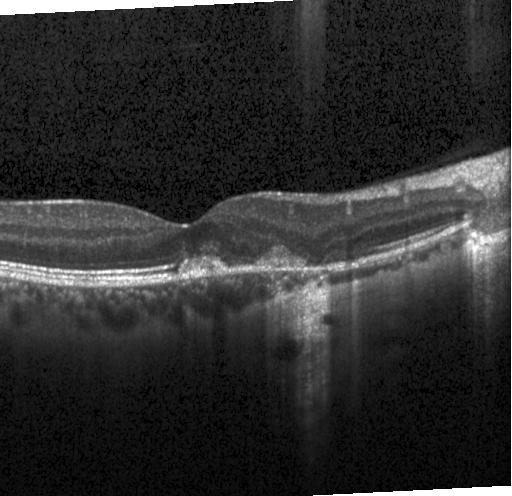 Diagnosis: choroidal neovascularization (CNV).